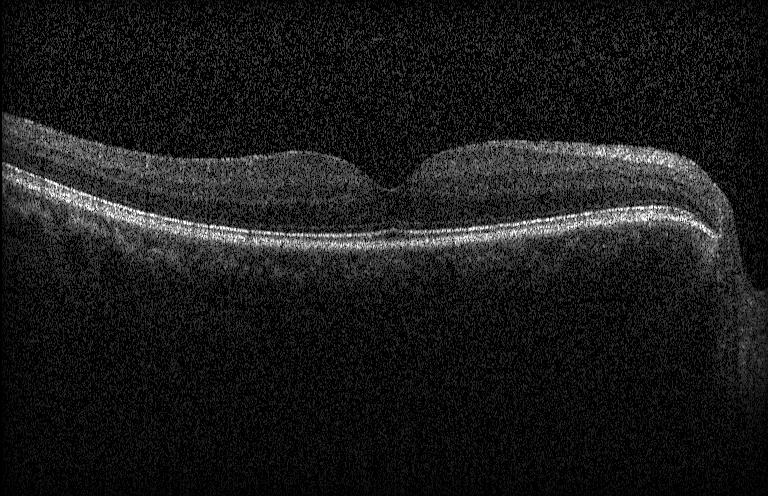

Optical coherence tomography B-scan; Heidelberg Spectralis
Impression: neither choroidal neovascularization, diabetic macular edema, nor drusen.